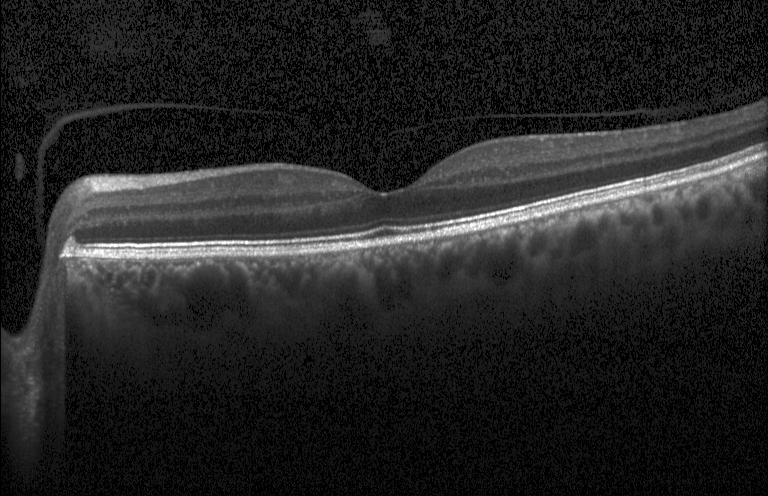
Finding: neither choroidal neovascularization, diabetic macular edema, nor drusen.